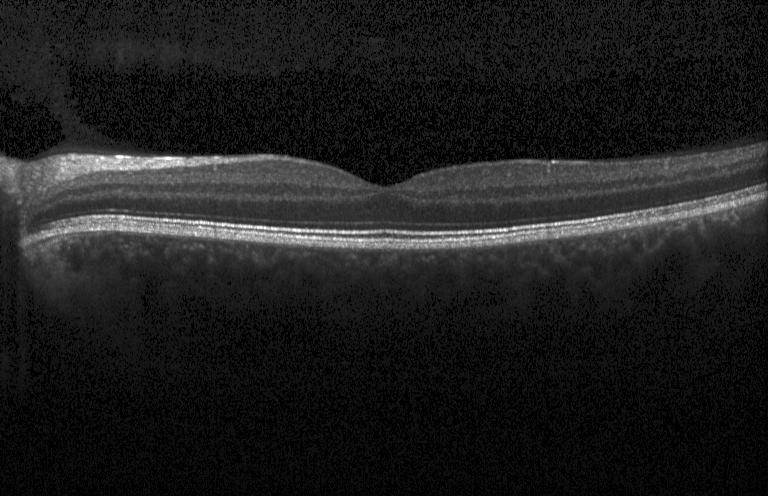 Horizontal scan through the fovea; spectral-domain OCT; optical coherence tomography B-scan.
Diagnosis: no evidence of choroidal neovascularization, diabetic macular edema, or drusen.